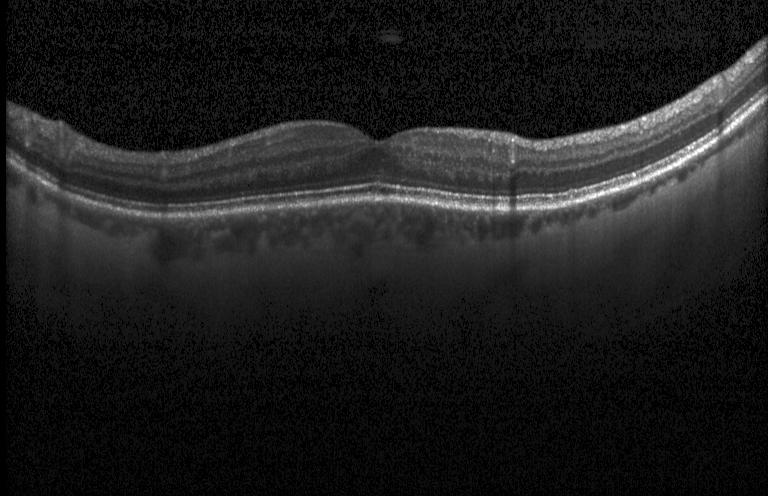 Diagnosis: neither choroidal neovascularization, diabetic macular edema, nor drusen.